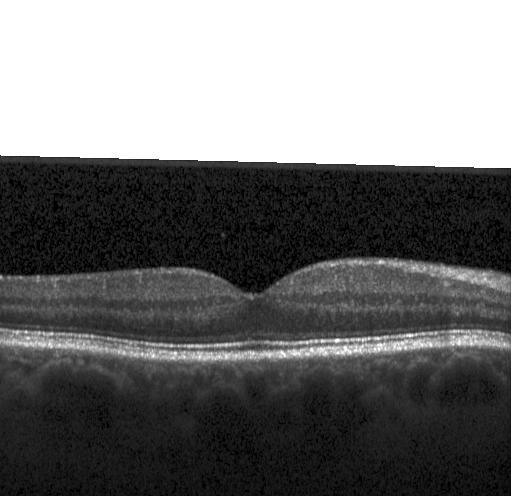

Spectral-domain optical coherence tomography · optical coherence tomography scan · through the macula.
Finding: no choroidal neovascularization, diabetic macular edema, or drusen.